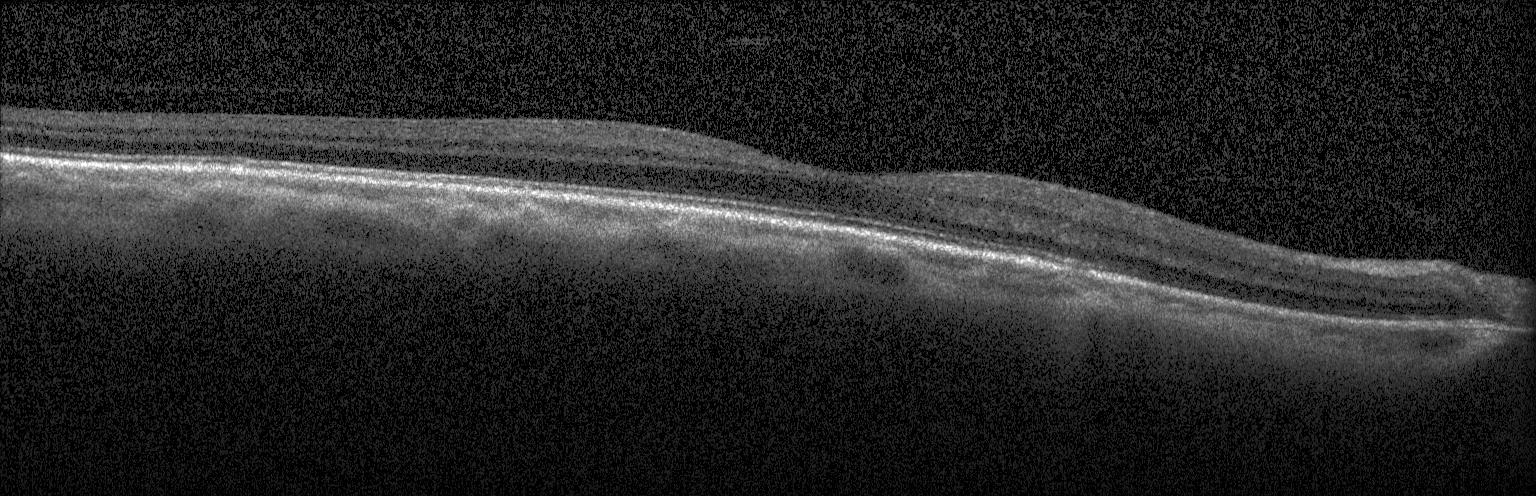
Heidelberg Spectralis OCT system. Macular scan. OCT B-scan. Spectral-domain optical coherence tomography
Assessment: no choroidal neovascularization, diabetic macular edema, or drusen.